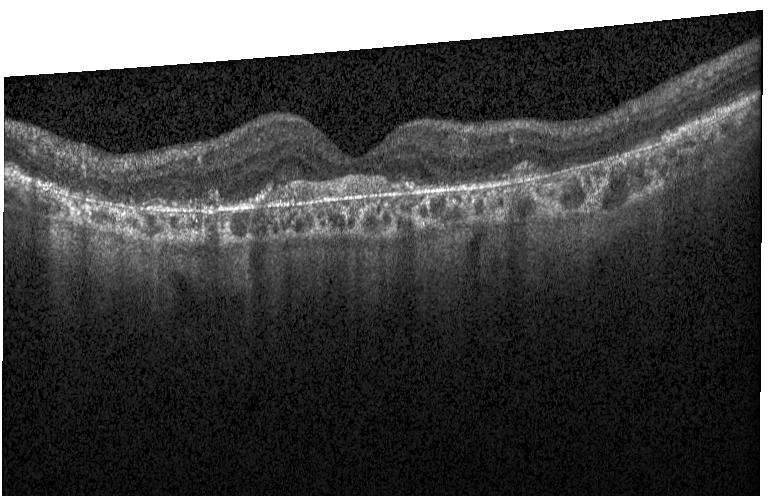

Optical coherence tomography scan; centered on the fovea; spectral-domain optical coherence tomography — Diagnosis: CNV.